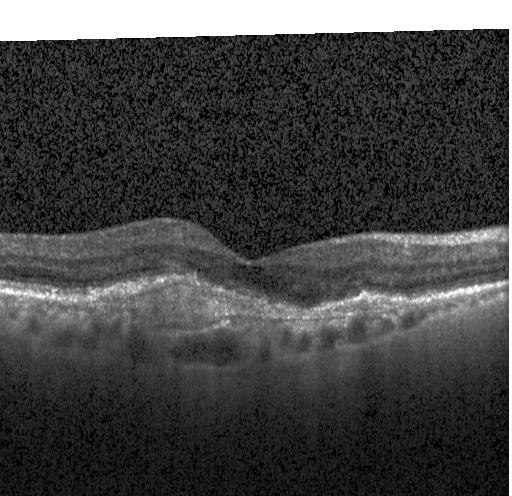

Macular OCT: choroidal neovascularization.